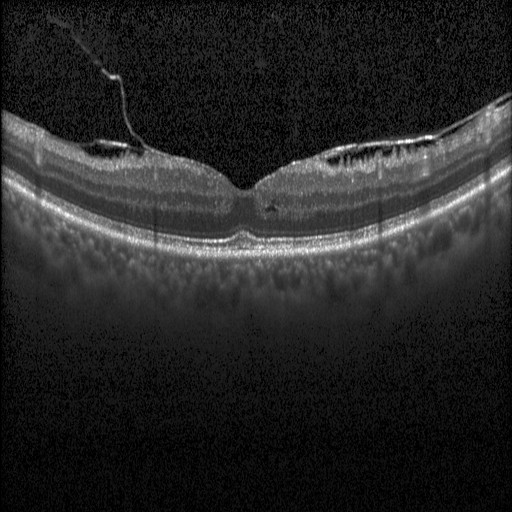
Spectral-domain OCT · centered on the fovea · Heidelberg Spectralis · OCT B-scan. Dx: diabetic macular edema.